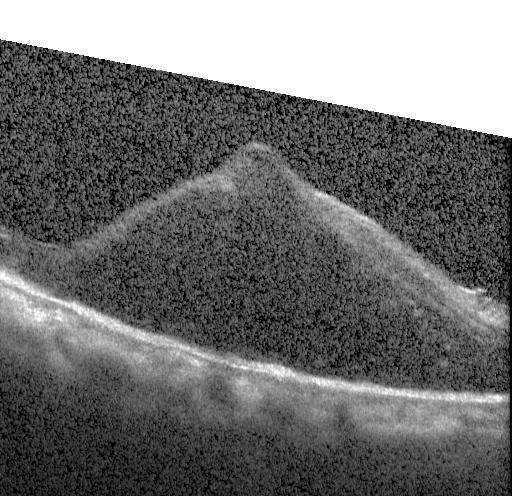

Dx: diabetic macular edema (DME).